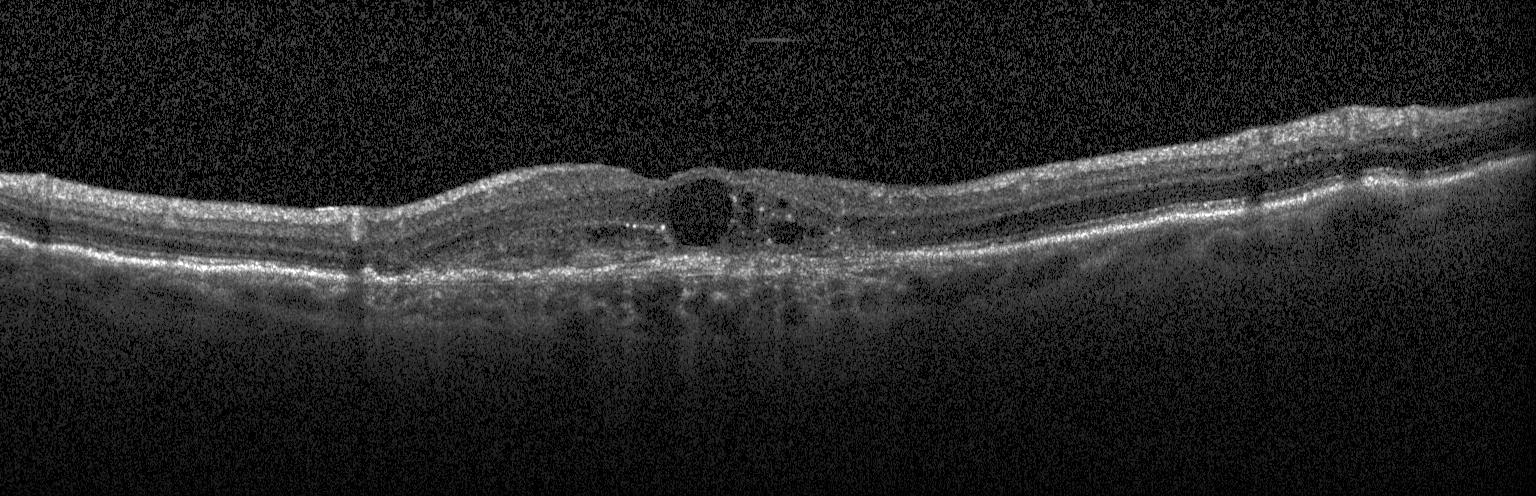
OCT B-scan.
OCT finding: CNV.